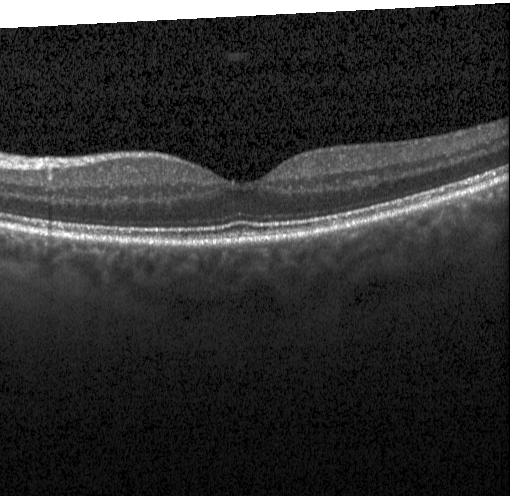 OCT B-scan. Spectral-domain OCT. Horizontal scan through the fovea — Assessment: no choroidal neovascularization, no diabetic macular edema, and no drusen.